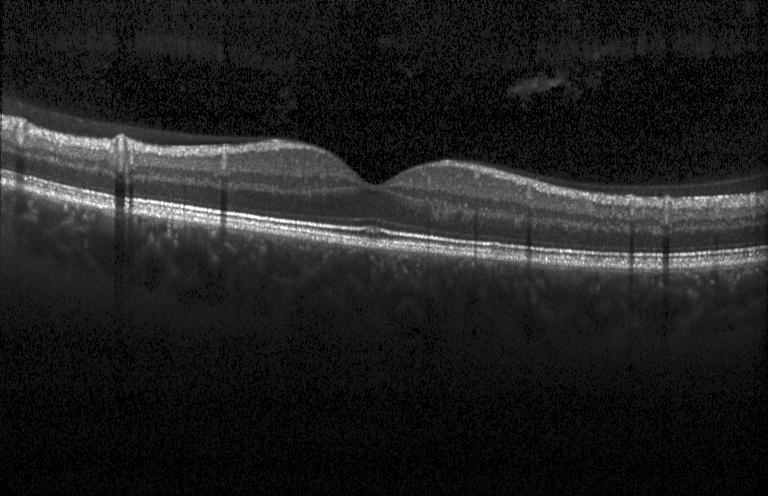 OCT line scan.
Diagnosis: no CNV, no DME, and no drusen.